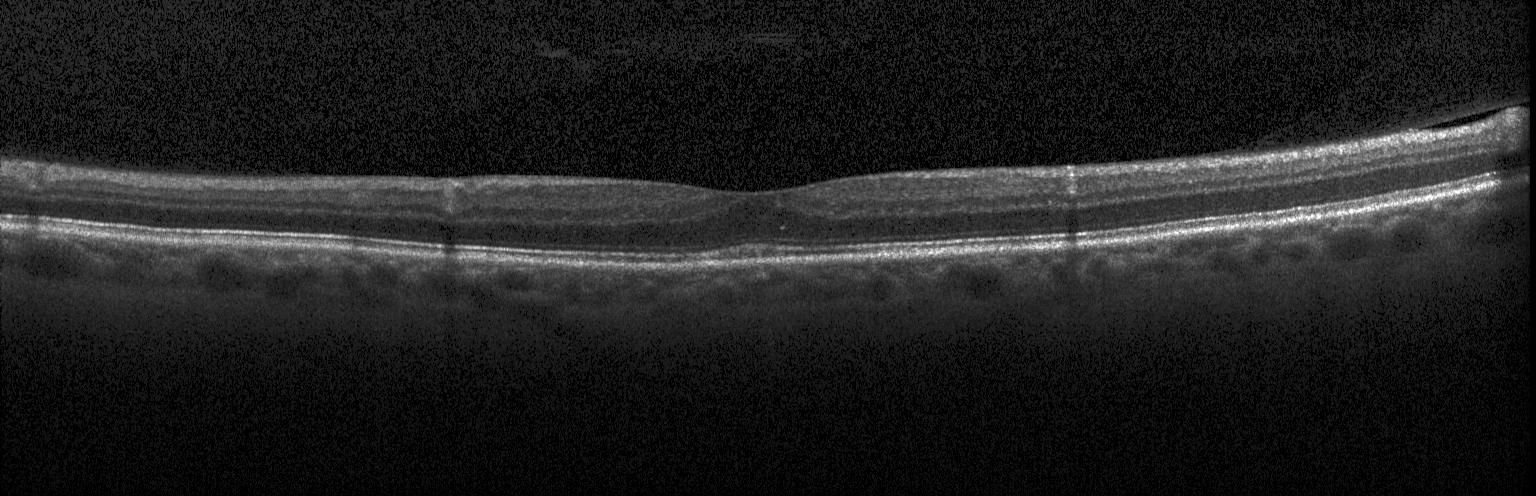 OCT line scan; through the macula; acquired on a Heidelberg Spectralis; spectral-domain optical coherence tomography. Impression: no choroidal neovascularization, diabetic macular edema, or drusen.